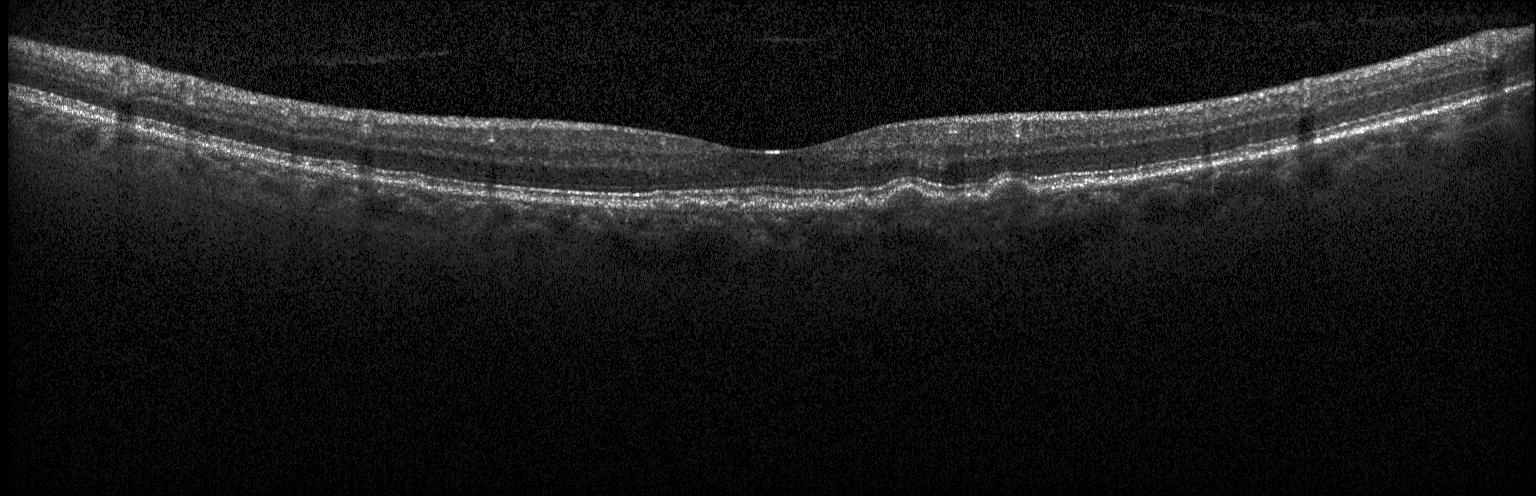

Heidelberg Spectralis, fovea-centered, OCT line scan.
Finding: sub-RPE drusenoid deposits.